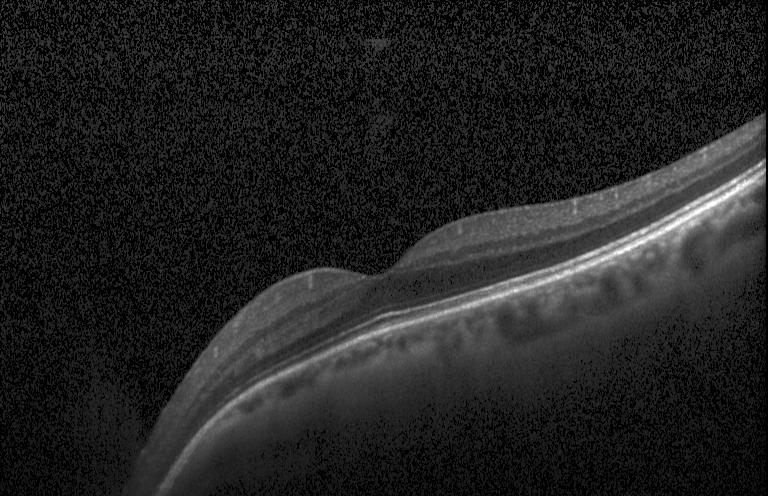
Heidelberg Spectralis, horizontal scan through the fovea, spectral-domain OCT, retinal OCT B-scan — The scan shows no choroidal neovascularization, diabetic macular edema, or drusen.